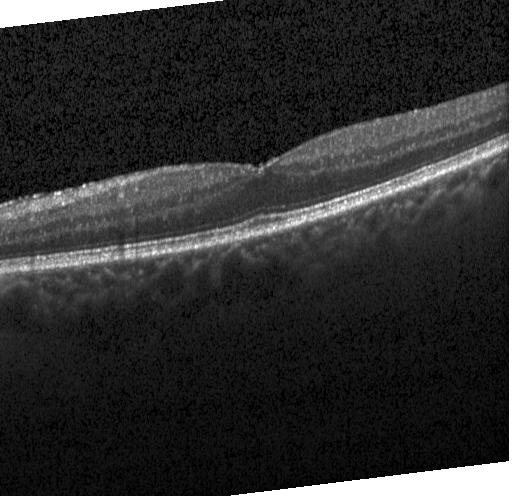
The scan shows no evidence of CNV, DME, or drusen.